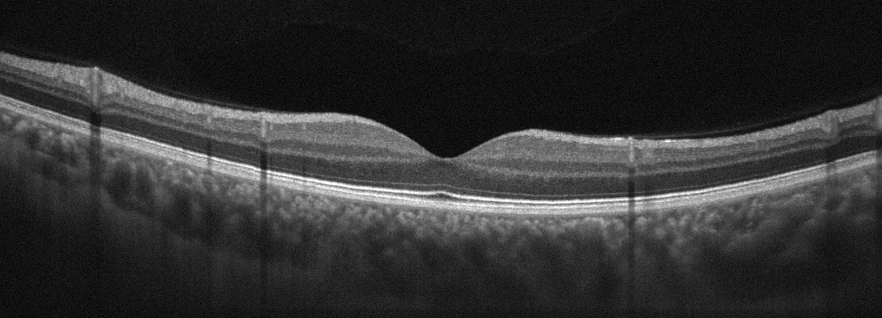 OD · optical coherence tomography B-scan. Diagnosis: absence of AMD, DME, ERM, RAO, RVO, and vitreomacular interface disease.